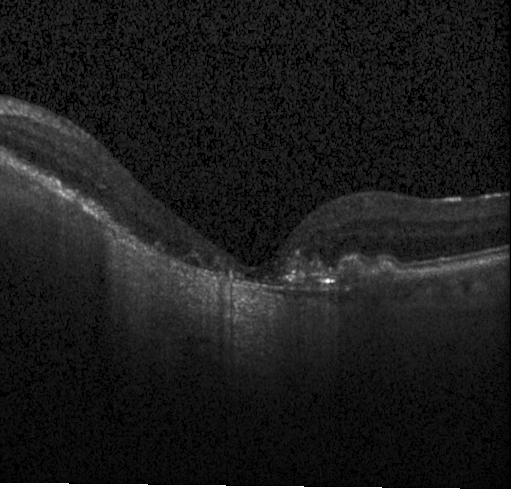 Spectral-domain optical coherence tomography. Optical coherence tomography scan. Horizontal scan through the fovea. Heidelberg Spectralis — This B-scan demonstrates choroidal neovascularization (CNV).